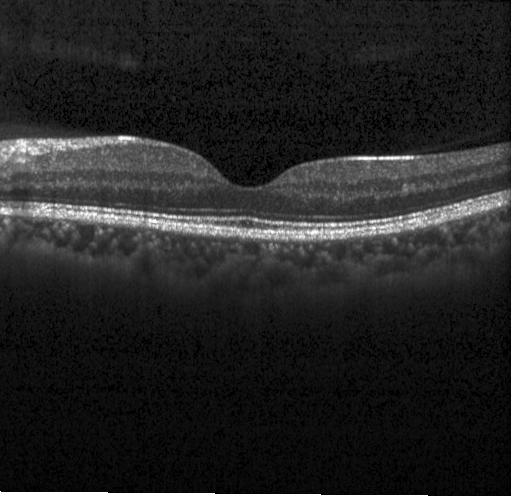
Finding: no choroidal neovascularization, no diabetic macular edema, and no drusen.